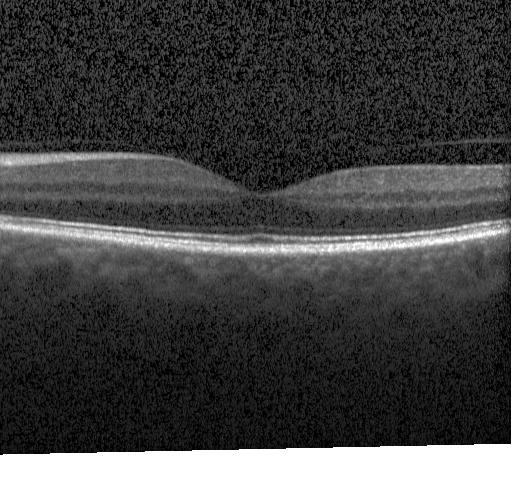

OCT B-scan, Heidelberg Spectralis OCT system — Impression: no choroidal neovascularization, no diabetic macular edema, and no drusen.